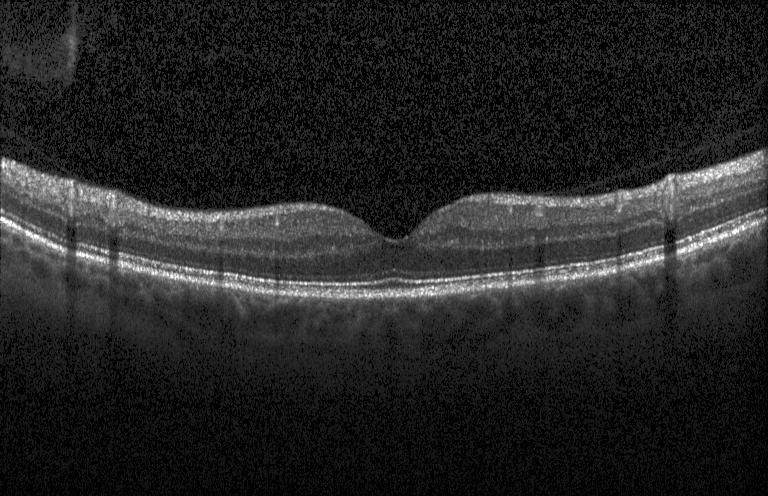
SD-OCT, retinal OCT B-scan, macular scan
Diagnosis: no CNV, no DME, and no drusen.